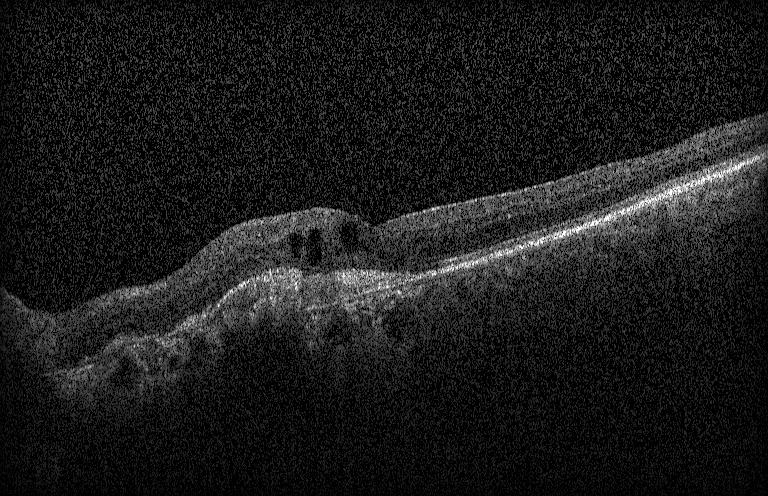
OCT scan showing a choroidal neovascular membrane.